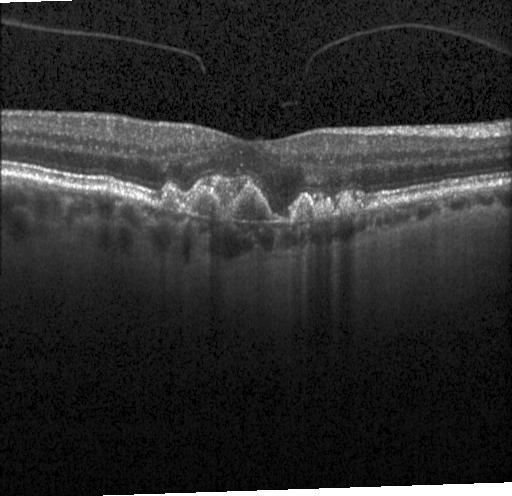 Diagnosis: a choroidal neovascular membrane.